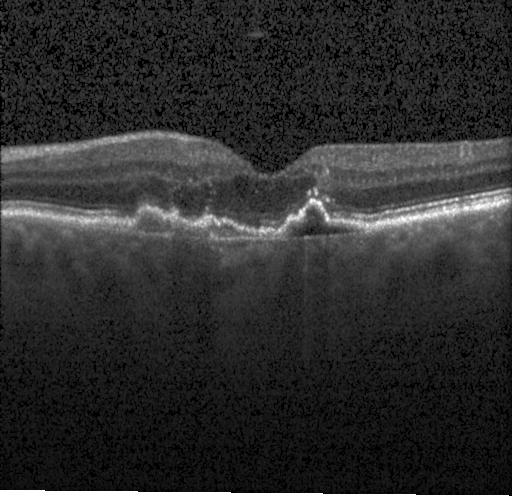
Centered on the fovea. Optical coherence tomography B-scan
Dx: a choroidal neovascular membrane.